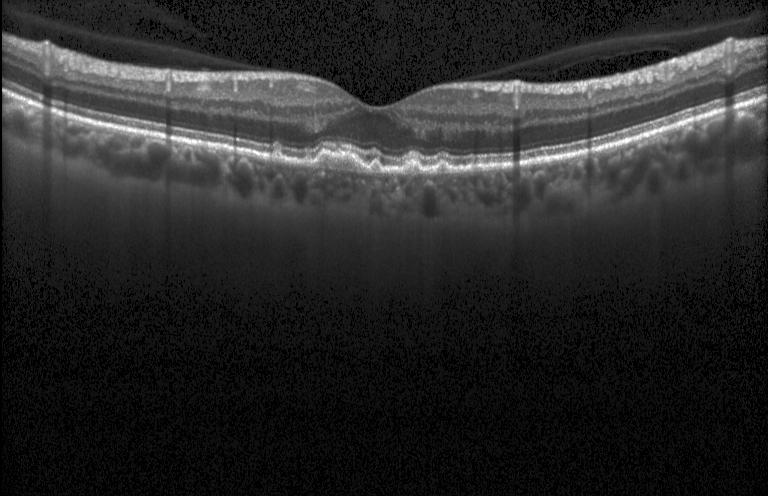 Fovea-centered. Spectral-domain optical coherence tomography. Heidelberg Spectralis. OCT B-scan.
The scan shows multiple drusen.